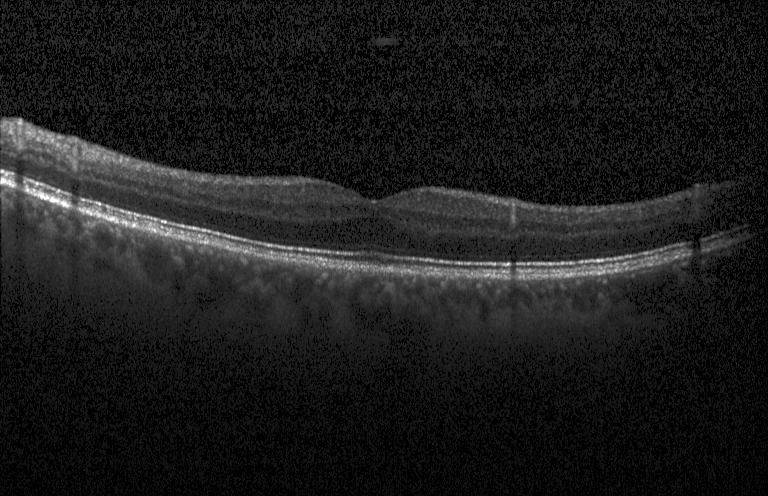

Optical coherence tomography B-scan. Spectral-domain OCT
Finding: no evidence of choroidal neovascularization, diabetic macular edema, or drusen.